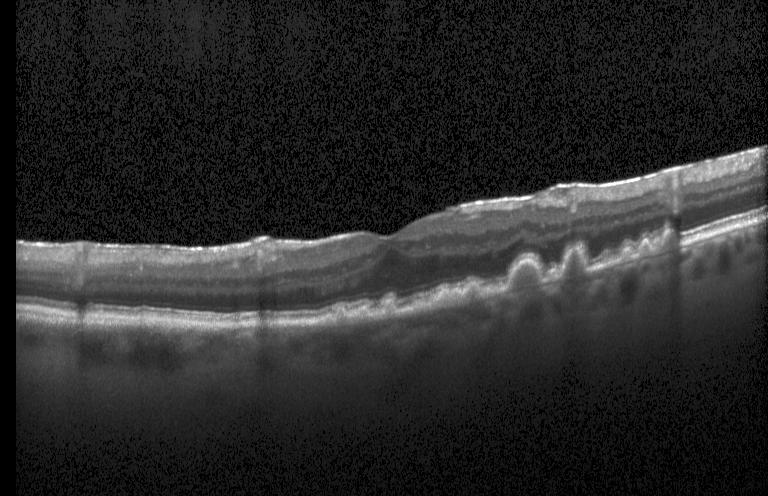 Retinal OCT B-scan. Horizontal scan through the fovea. Spectral-domain OCT. Impression: sub-RPE drusenoid deposits.